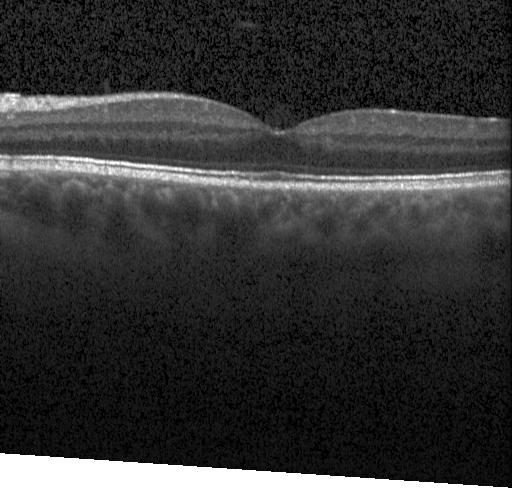 OCT B-scan; fovea-centered; Heidelberg Spectralis.
No evidence of choroidal neovascularization, diabetic macular edema, or drusen.